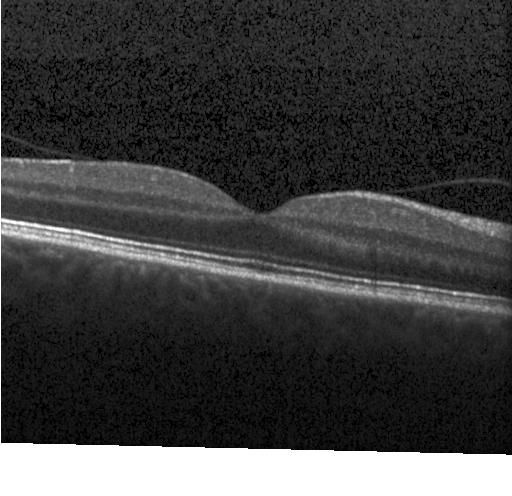

Dx: neither CNV, DME, nor drusen.